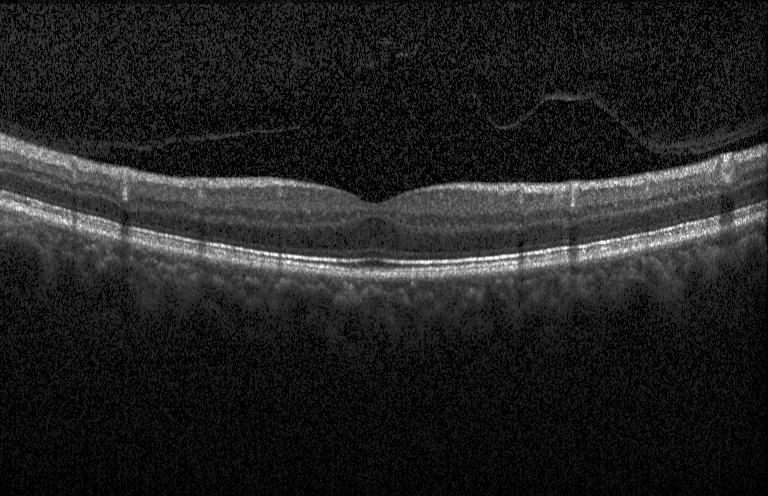 OCT scan showing no choroidal neovascularization, diabetic macular edema, or drusen.